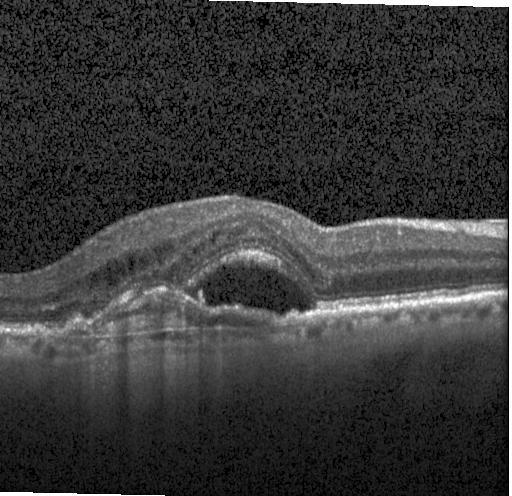

Fovea-centered. Optical coherence tomography B-scan.
Diagnosis: choroidal neovascularization (CNV).